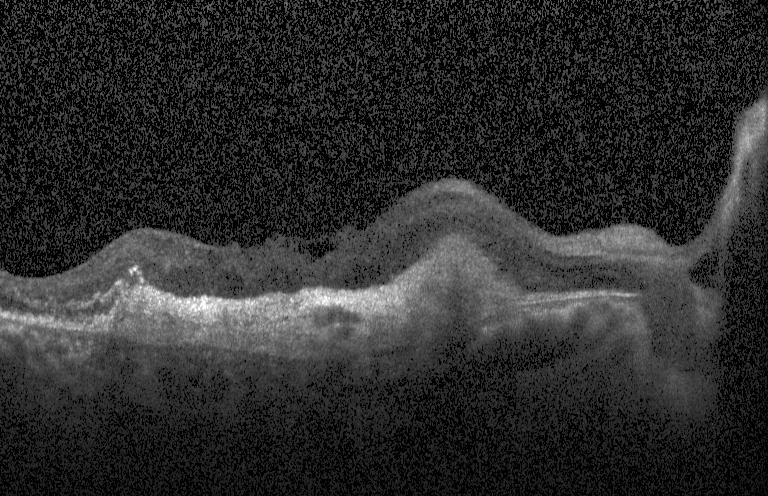

Choroidal neovascularization (CNV).